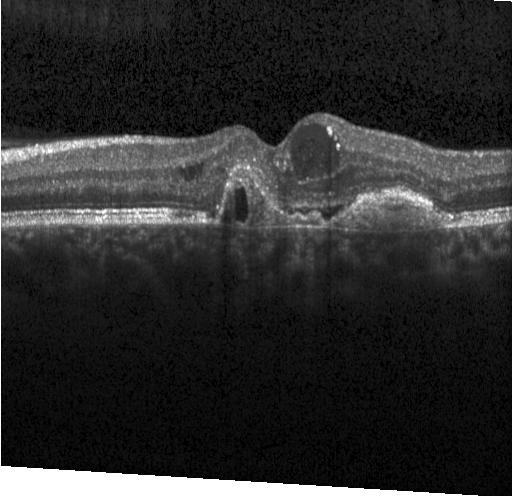
OCT B-scan. Finding: choroidal neovascularization (CNV).